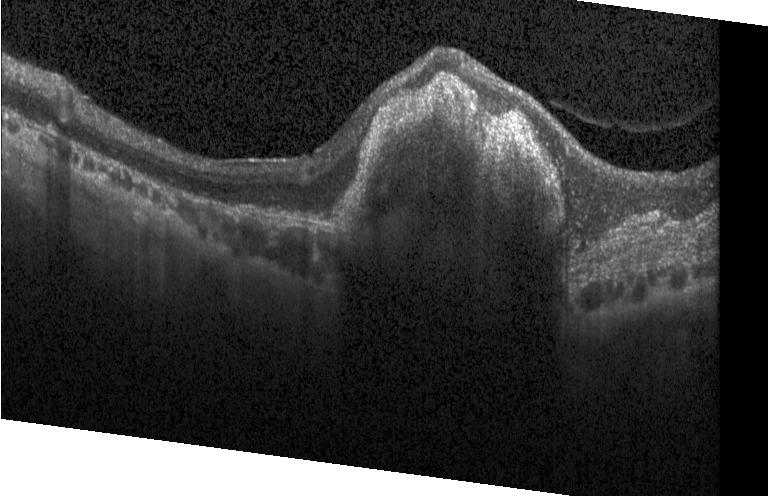
Heidelberg Spectralis OCT system · retinal OCT B-scan · SD-OCT · through the macula — Macular OCT: a choroidal neovascular membrane.